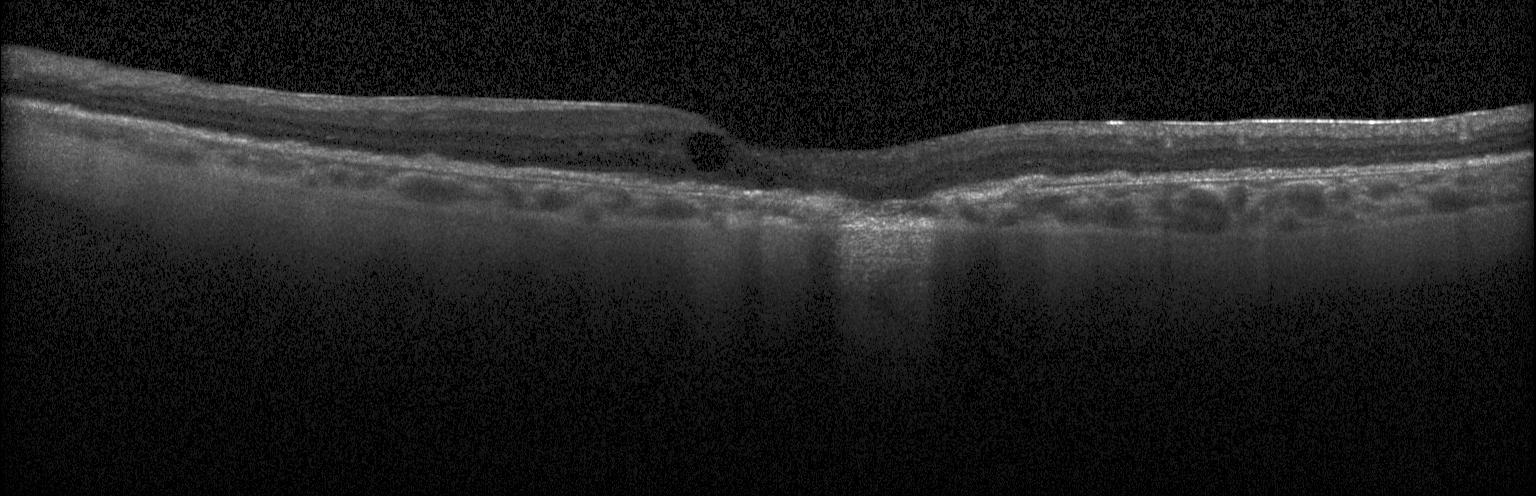
CNV.